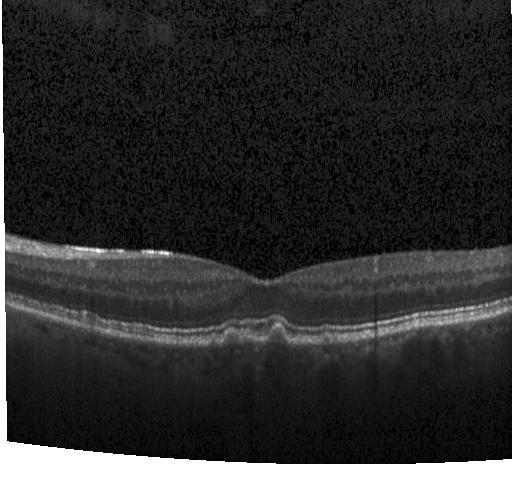 OCT B-scan · centered on the fovea · acquired on a Heidelberg Spectralis — Sub-RPE drusenoid deposits.